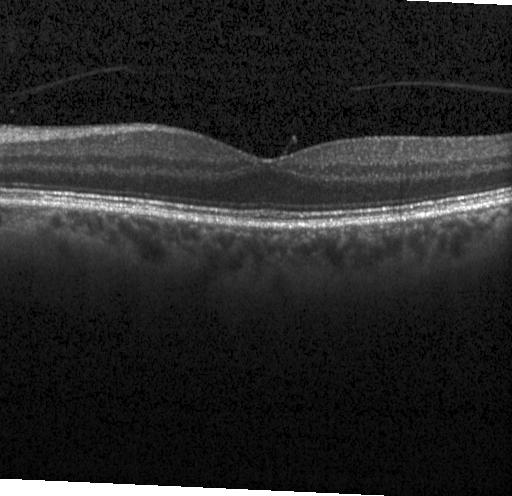 Centered on the fovea, OCT B-scan, acquired on a Heidelberg Spectralis.
Assessment: no choroidal neovascularization, no diabetic macular edema, and no drusen.